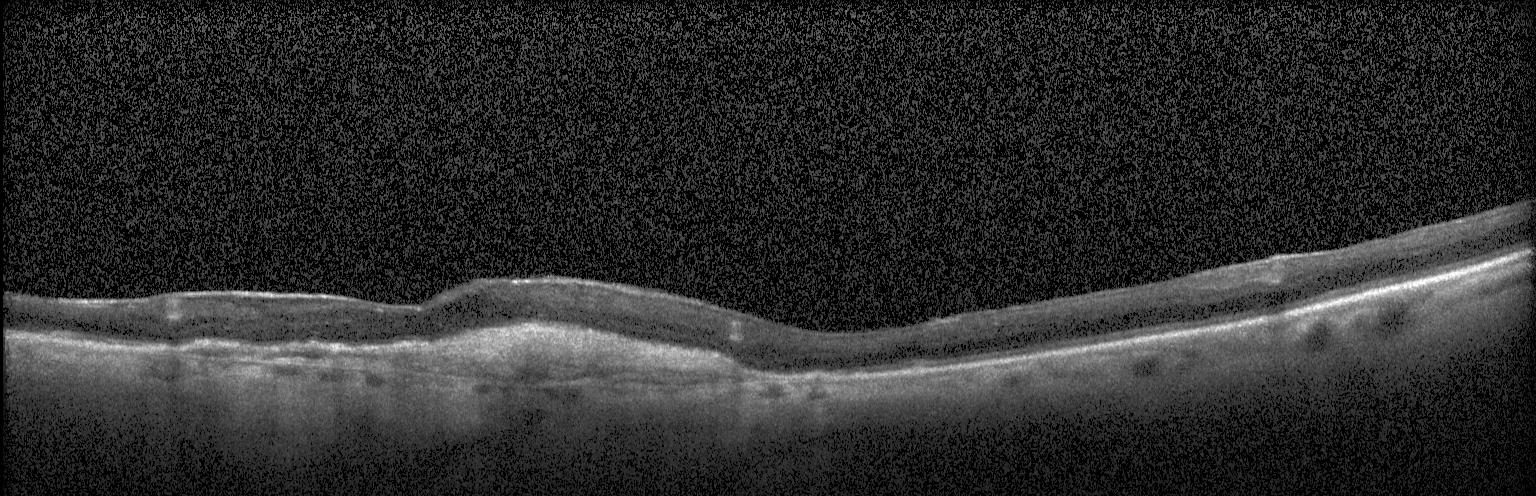
Optical coherence tomography B-scan
Macular OCT: choroidal neovascularization (CNV).